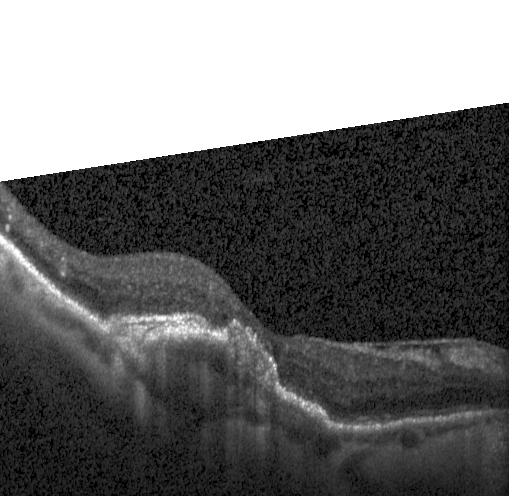

Diagnosis: choroidal neovascularization.